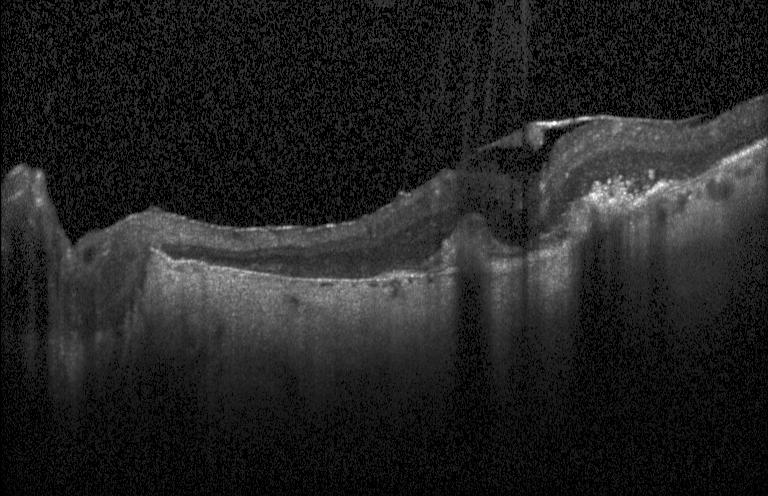 Macular OCT demonstrating a choroidal neovascular membrane.